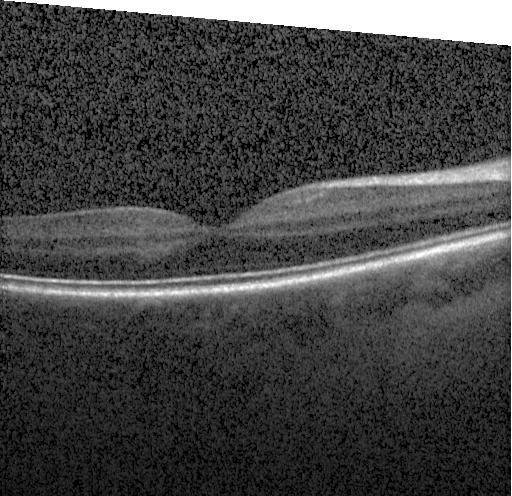

OCT line scan, acquired on a Heidelberg Spectralis. Impression: neither choroidal neovascularization, diabetic macular edema, nor drusen.